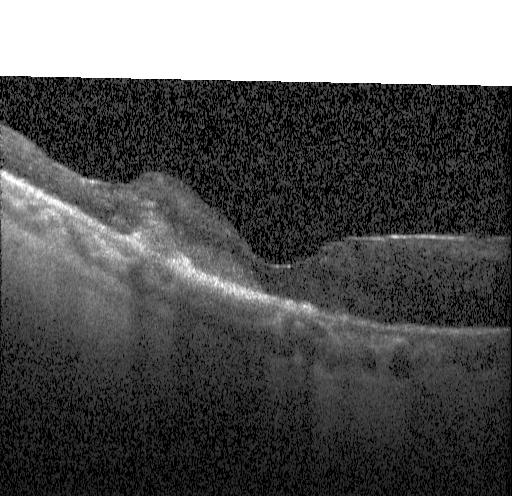
OCT line scan, SD-OCT.
OCT finding: a choroidal neovascular membrane.